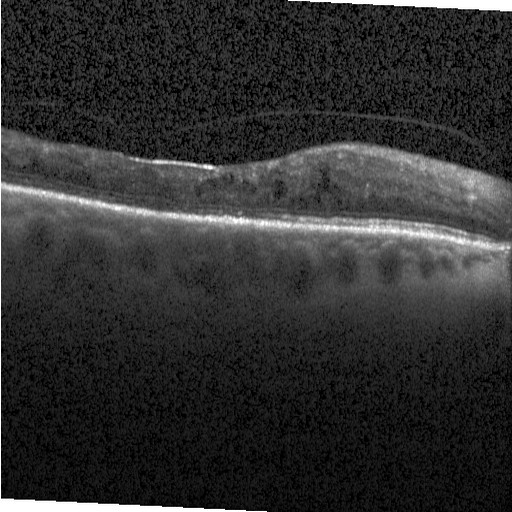
Finding: DME.